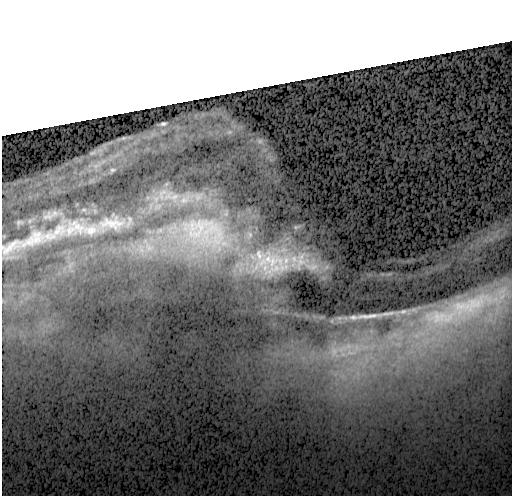

Acquired on a Heidelberg Spectralis, spectral-domain OCT, OCT line scan.
Impression: a choroidal neovascular membrane.